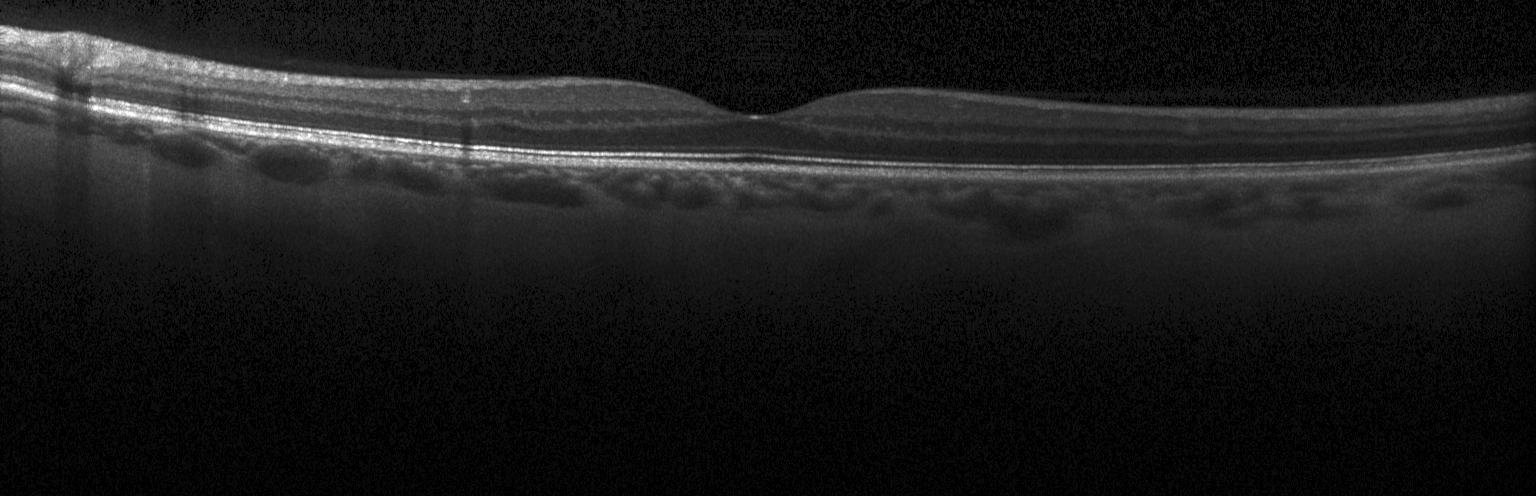

Dx: no evidence of choroidal neovascularization, diabetic macular edema, or drusen.